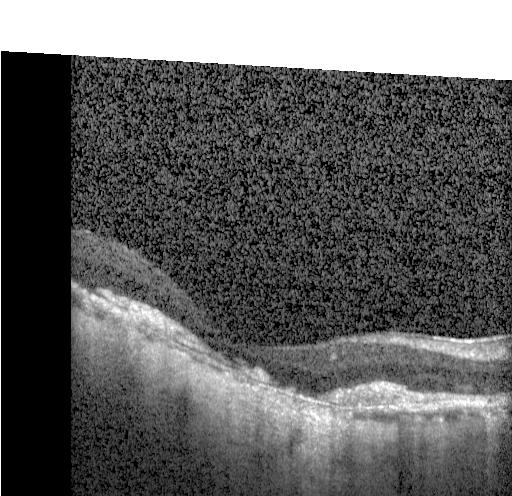 Spectral-domain optical coherence tomography. Heidelberg Spectralis OCT system. OCT B-scan. Horizontal scan through the fovea.
Dx: CNV.